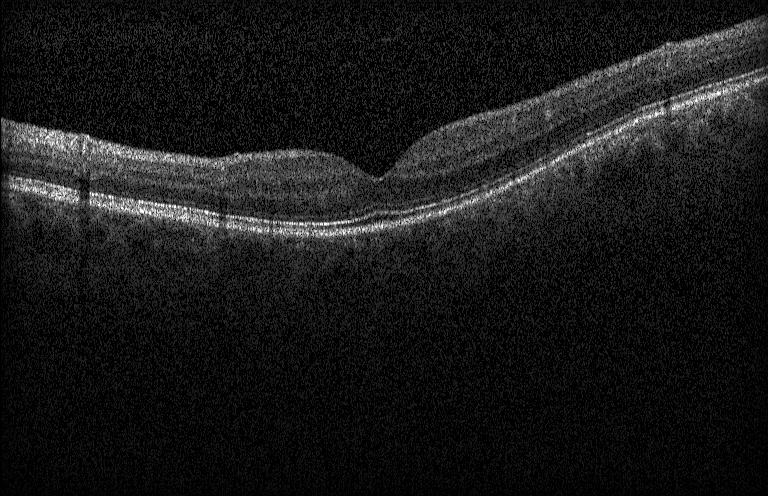
Finding: no evidence of CNV, DME, or drusen.